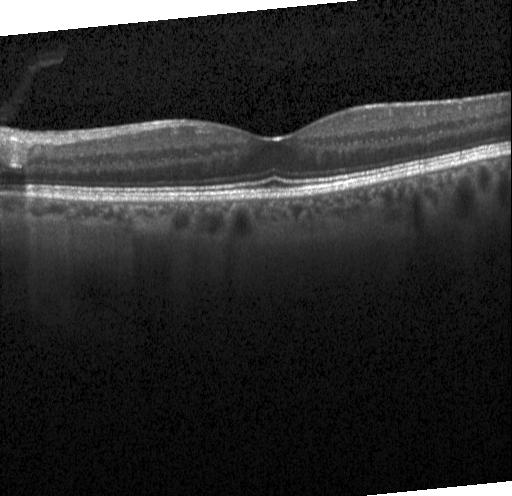
Spectral-domain optical coherence tomography; retinal OCT cross-section; instrument: Heidelberg Spectralis; fovea-centered. Diagnosis: no evidence of CNV, DME, or drusen.